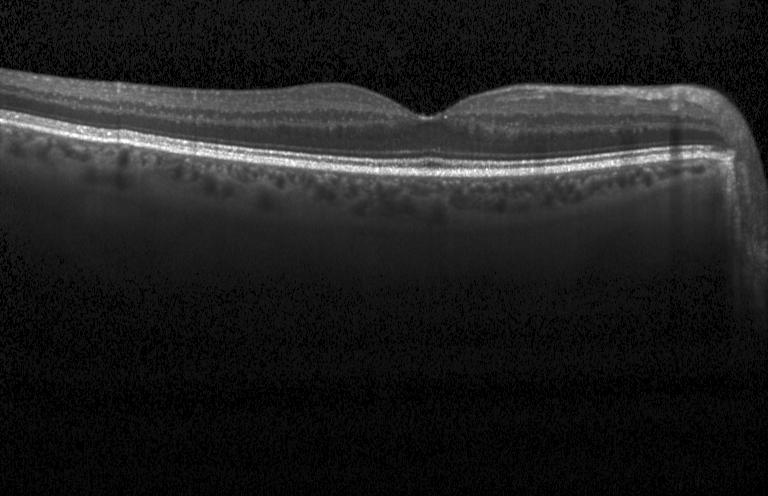
Retinal OCT cross-section · fovea-centered · Heidelberg Spectralis OCT system · SD-OCT.
Diagnosis: no CNV, DME, or drusen.